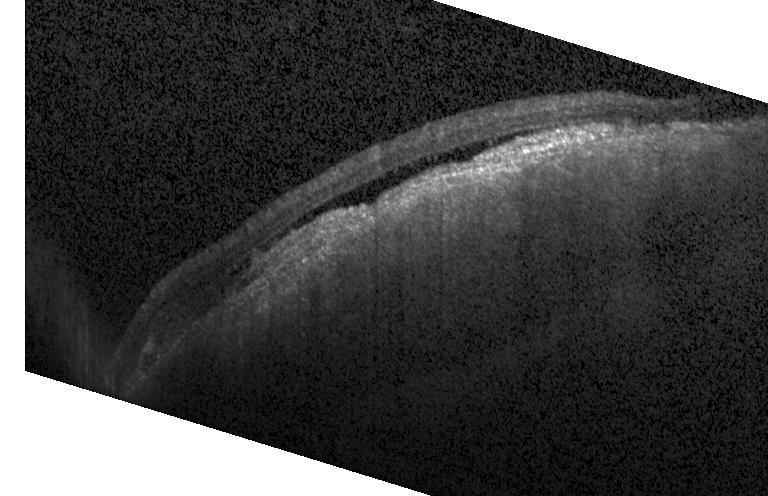
Acquired on a Heidelberg Spectralis; retinal OCT cross-section — Diagnosis: a choroidal neovascular membrane.